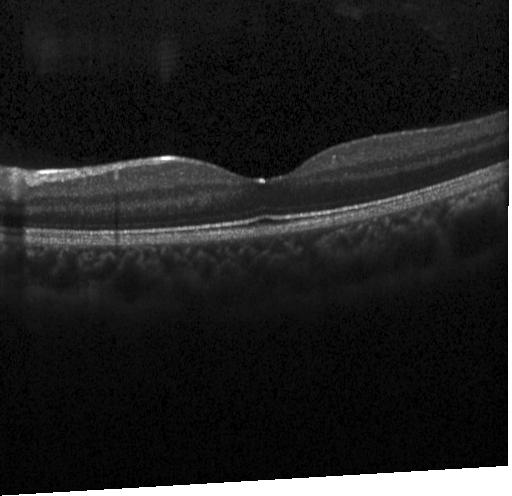 Spectral-domain OCT, through the macula, Heidelberg Spectralis OCT system, retinal OCT cross-section. Impression: no evidence of choroidal neovascularization, diabetic macular edema, or drusen.